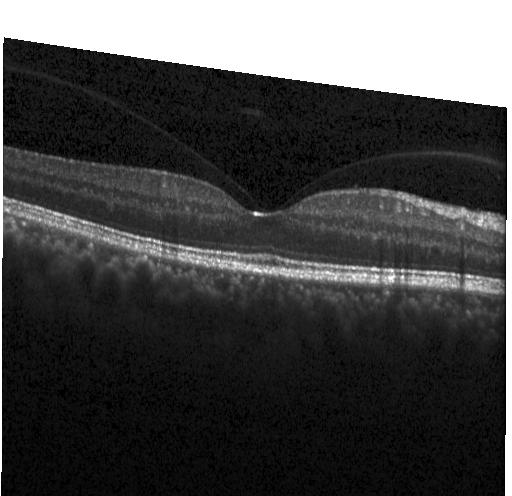

Diagnosis: no choroidal neovascularization, diabetic macular edema, or drusen.